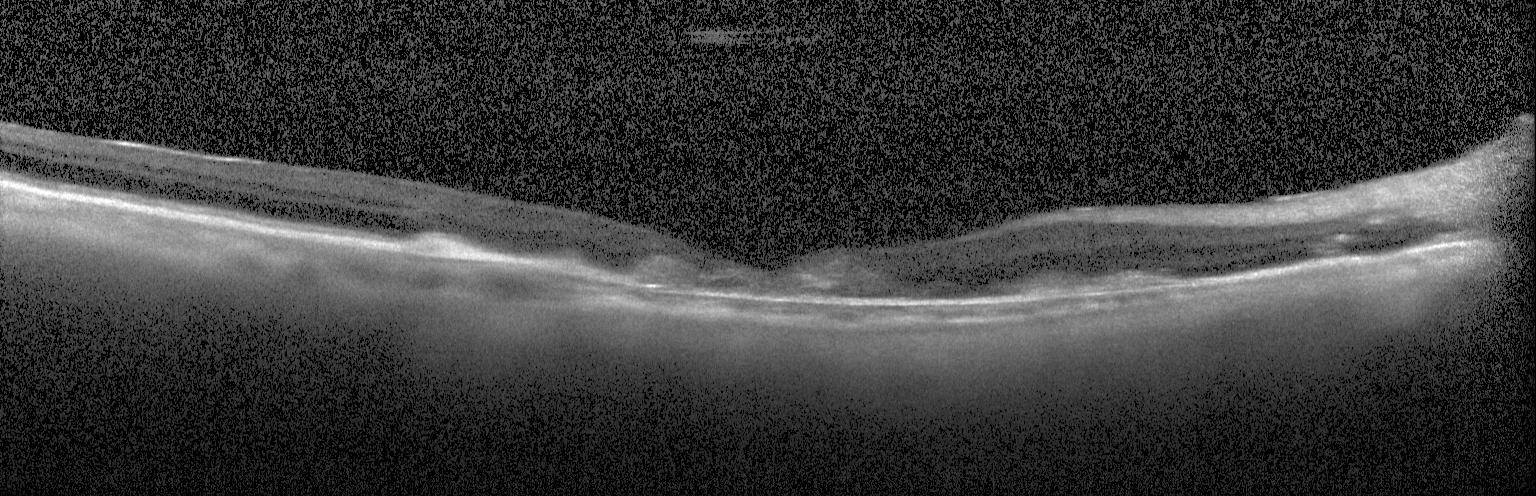

Finding: a choroidal neovascular membrane.